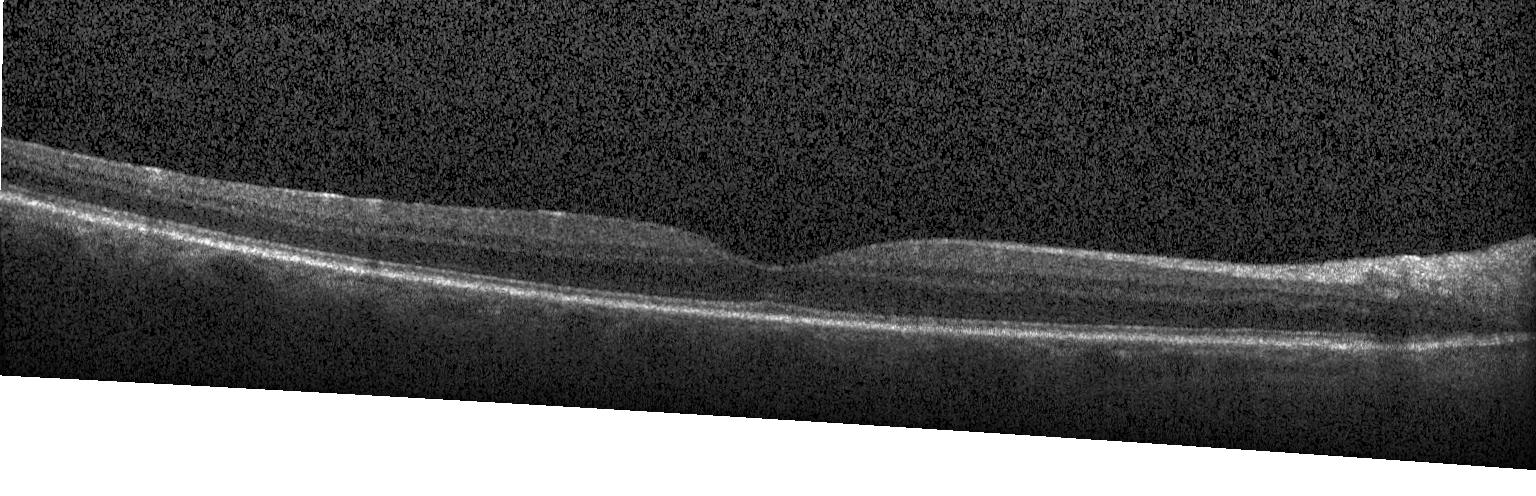 Retinal OCT cross-section
Neither choroidal neovascularization, diabetic macular edema, nor drusen.